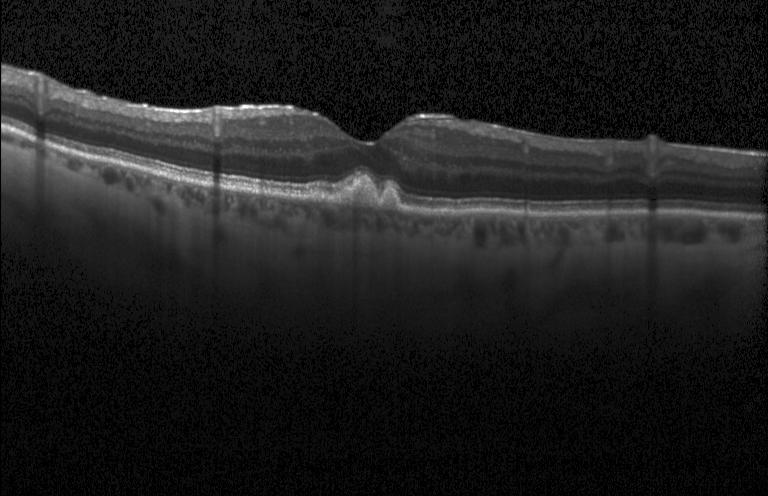 Optical coherence tomography scan. Impression: multiple drusen.